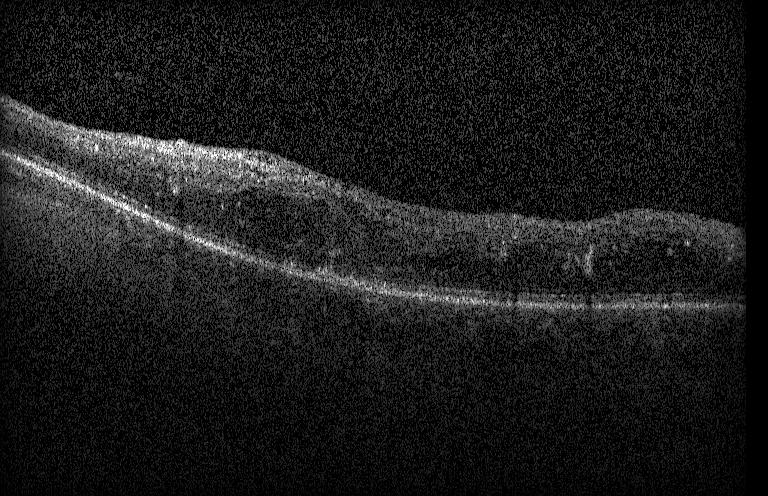
Dx: DME.